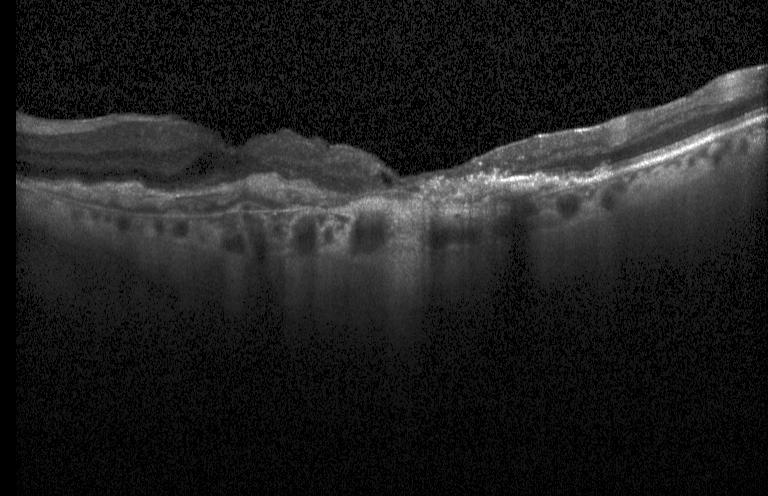

Impression: a choroidal neovascular membrane.